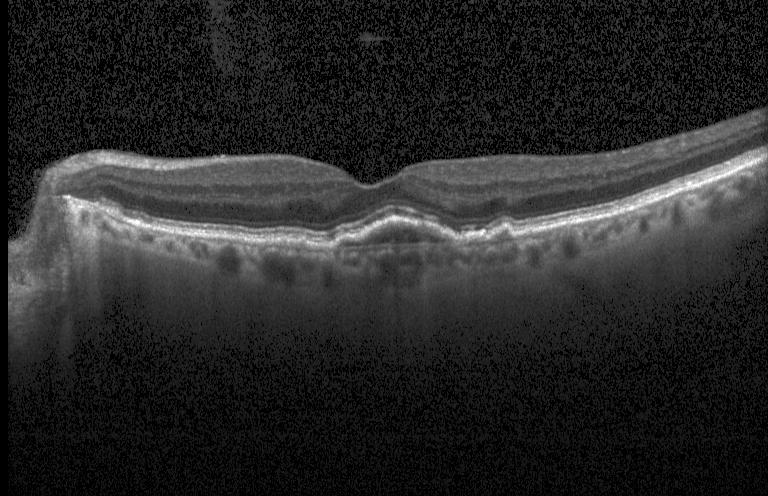
OCT scan showing a choroidal neovascular membrane.